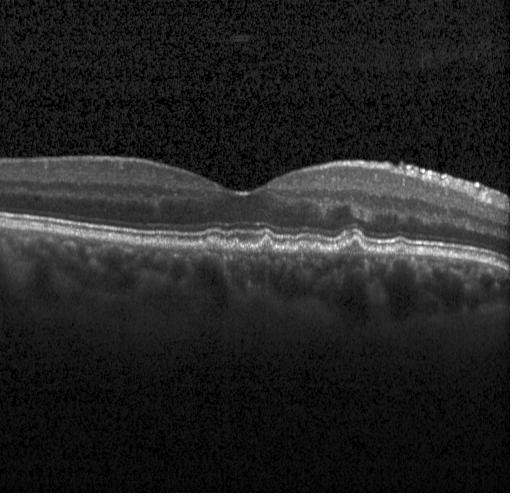

Retinal OCT cross-section. Diagnosis: drusen.